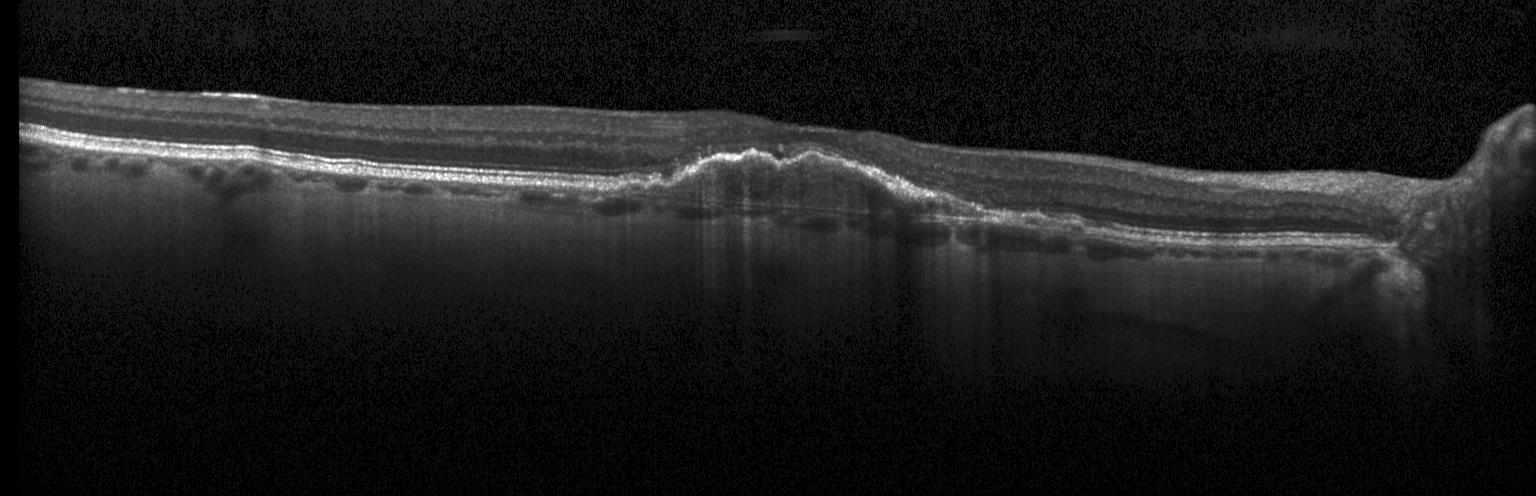

OCT finding: a choroidal neovascular membrane.